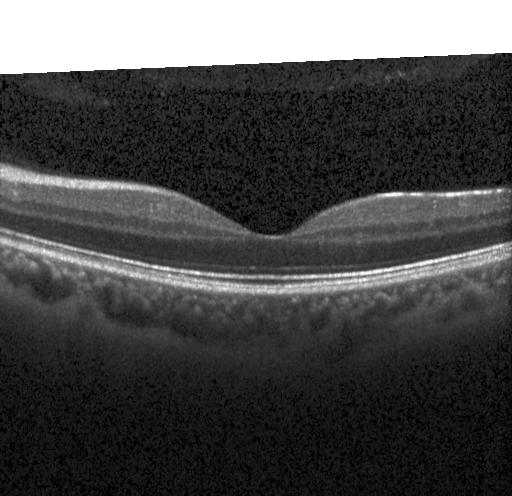

Neither CNV, DME, nor drusen.